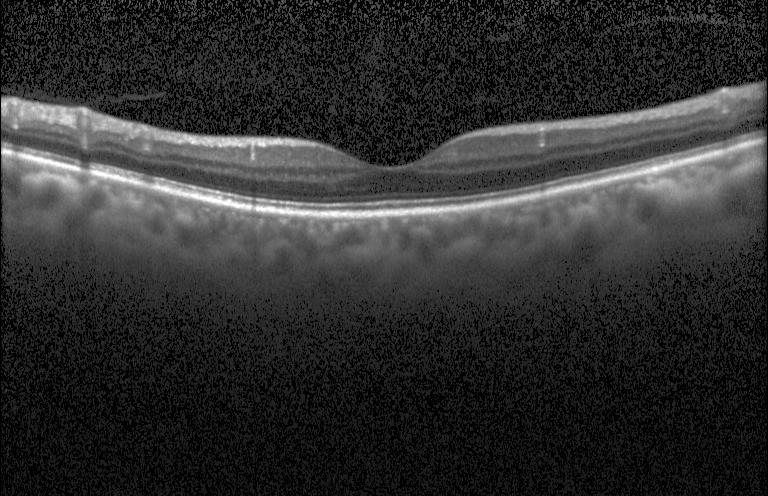

Assessment: neither choroidal neovascularization, diabetic macular edema, nor drusen.